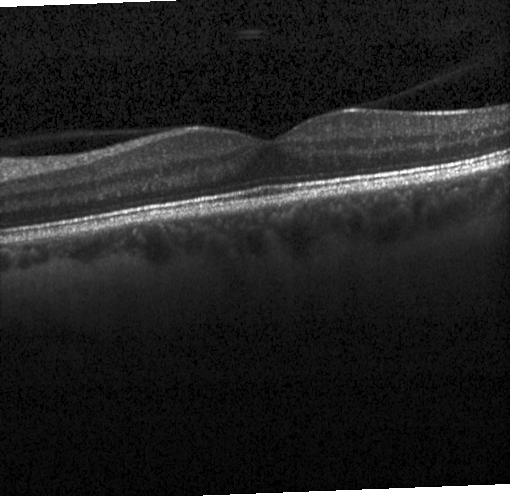
Heidelberg Spectralis OCT system; OCT line scan.
Diagnosis: no CNV, no DME, and no drusen.